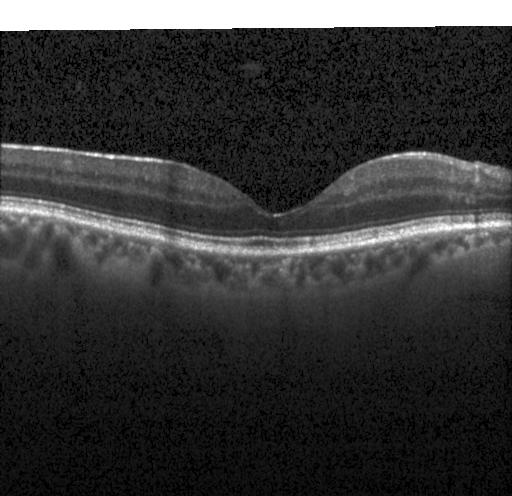 Macular OCT: no choroidal neovascularization, diabetic macular edema, or drusen.